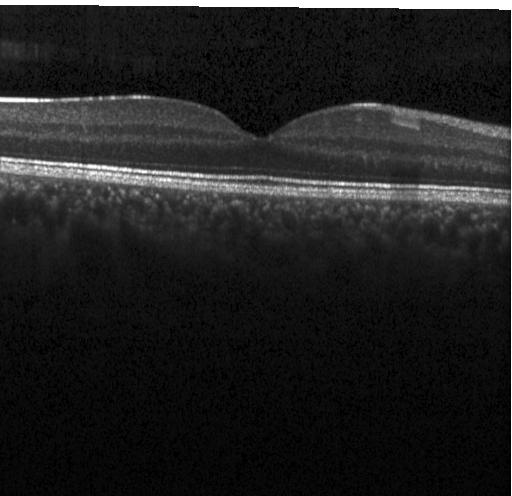 Finding: no choroidal neovascularization, no diabetic macular edema, and no drusen.